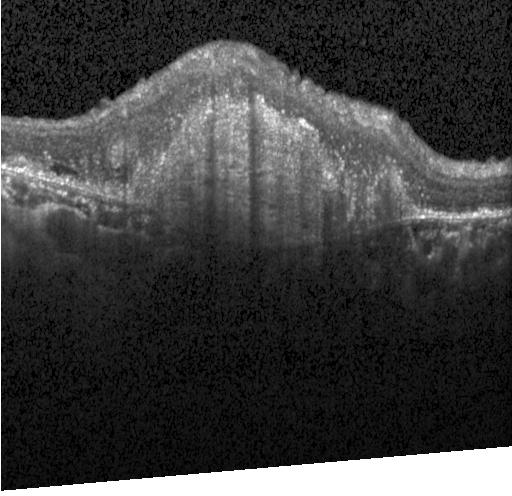
Optical coherence tomography B-scan
Macular OCT: CNV.